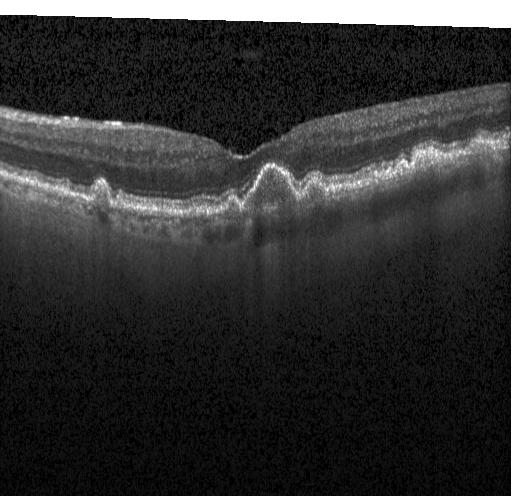 Macular scan, optical coherence tomography scan, acquired on a Heidelberg Spectralis — Finding: drusen.